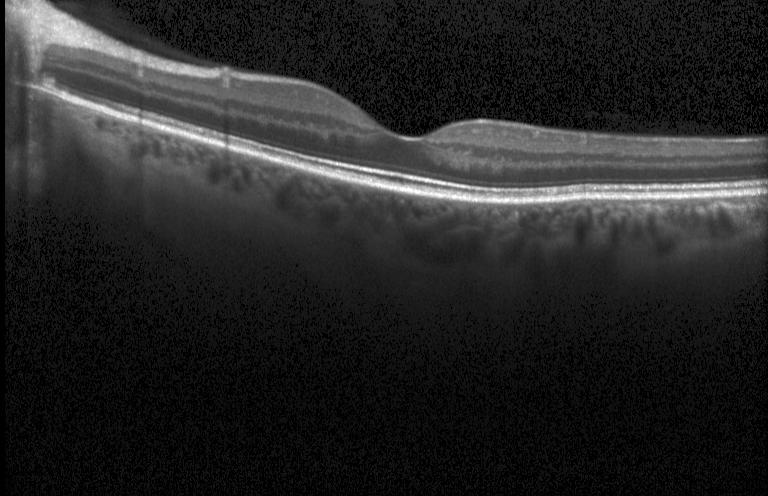
Retinal OCT B-scan, Heidelberg Spectralis OCT system
OCT finding: no choroidal neovascularization, diabetic macular edema, or drusen.